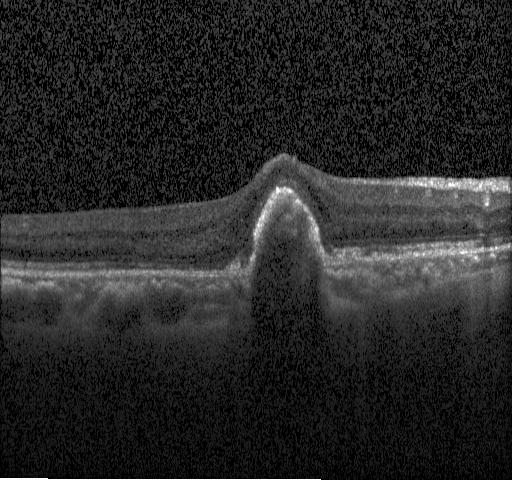 Fovea-centered; retinal OCT cross-section — Finding: choroidal neovascularization.